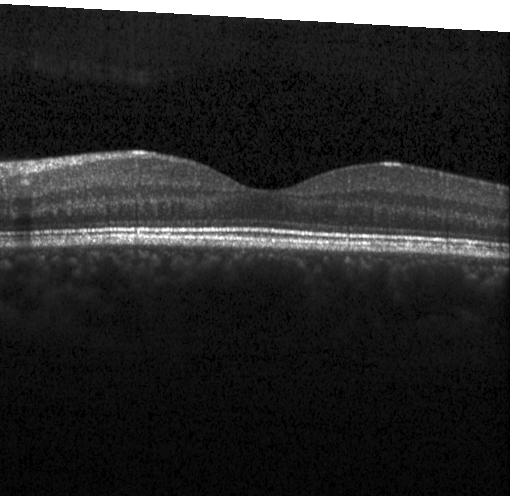 Acquired on a Heidelberg Spectralis, retinal OCT B-scan — Diagnosis: no CNV, DME, or drusen.